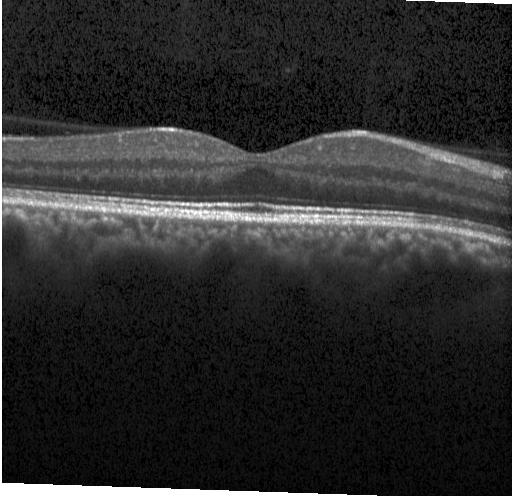

Spectral-domain optical coherence tomography; retinal OCT cross-section
Dx: no choroidal neovascularization, diabetic macular edema, or drusen.